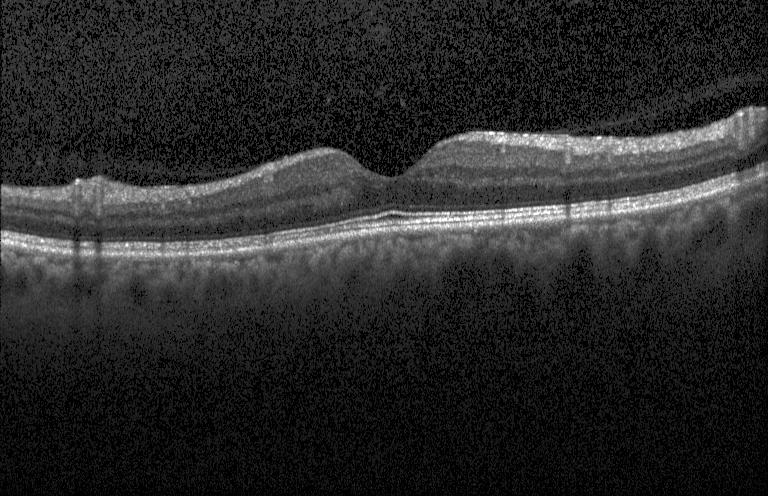
OCT line scan; spectral-domain optical coherence tomography; Heidelberg Spectralis; horizontal scan through the fovea
Impression: no choroidal neovascularization, no diabetic macular edema, and no drusen.